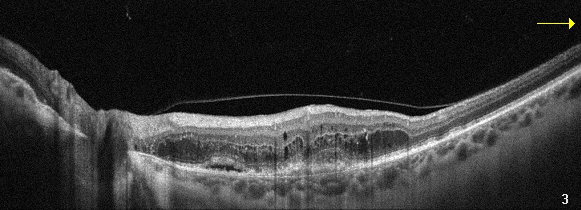
Diagnosis: age-related macular degeneration (AMD).